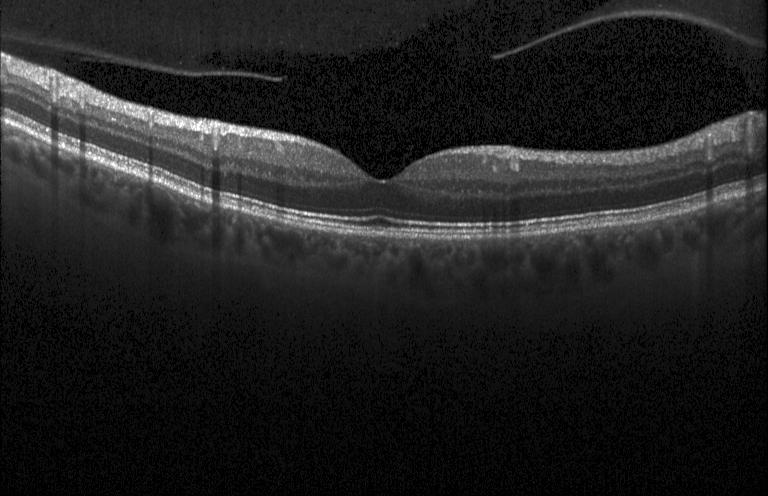
Retinal OCT B-scan. Dx: no choroidal neovascularization, no diabetic macular edema, and no drusen.